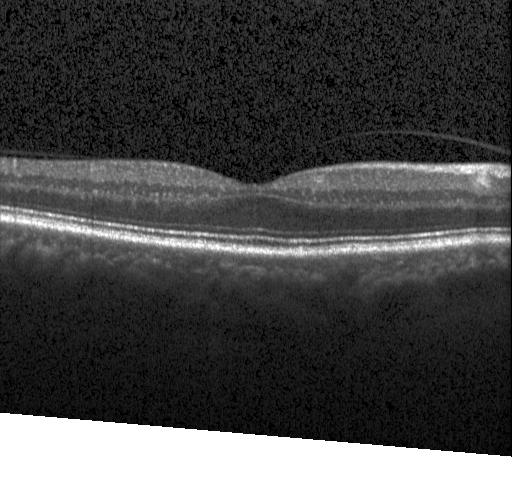
Optical coherence tomography B-scan
This B-scan demonstrates no choroidal neovascularization, diabetic macular edema, or drusen.